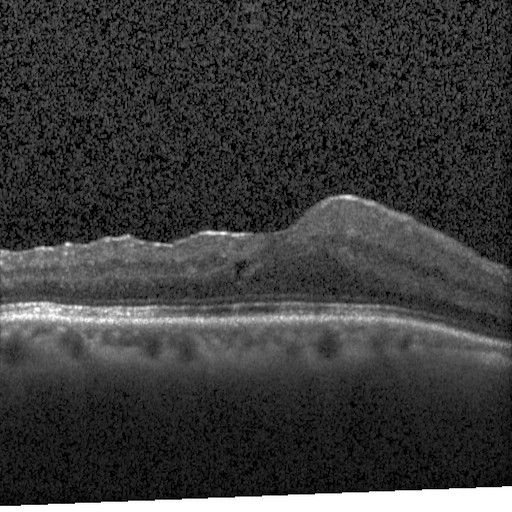

SD-OCT; fovea-centered; Heidelberg Spectralis; OCT B-scan — Finding: diabetic macular edema.